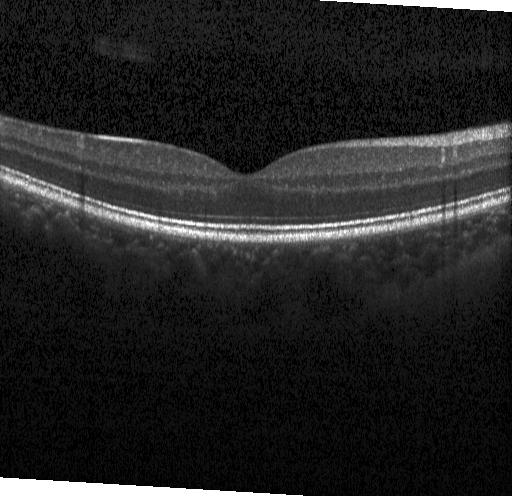 Diagnosis: neither choroidal neovascularization, diabetic macular edema, nor drusen.